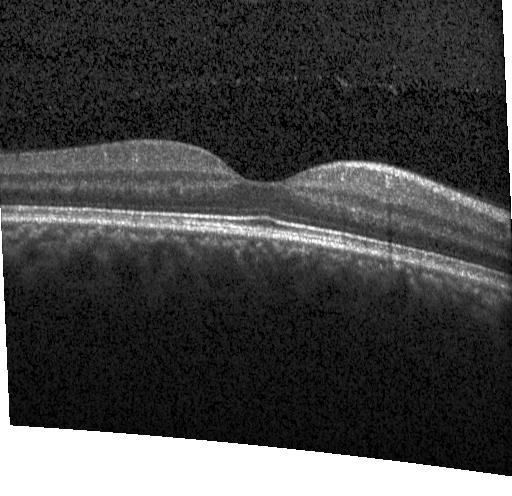

Centered on the fovea · retinal OCT cross-section · acquired on a Heidelberg Spectralis. No choroidal neovascularization, diabetic macular edema, or drusen.